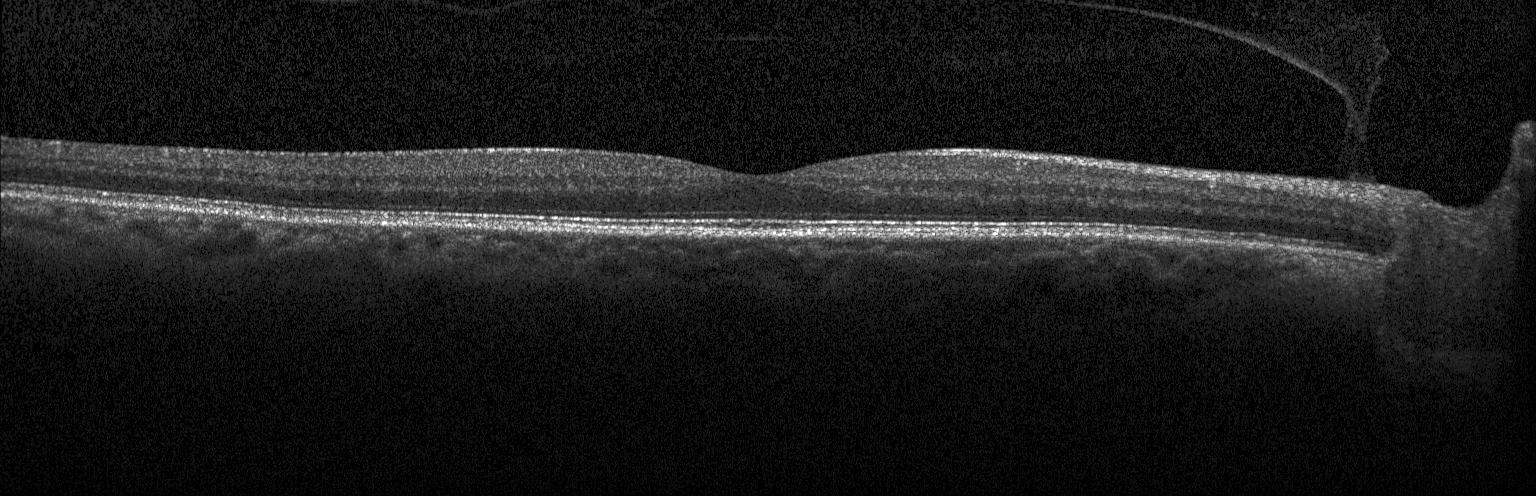 Macular scan; instrument: Heidelberg Spectralis; optical coherence tomography scan; spectral-domain optical coherence tomography. Impression: no CNV, DME, or drusen.